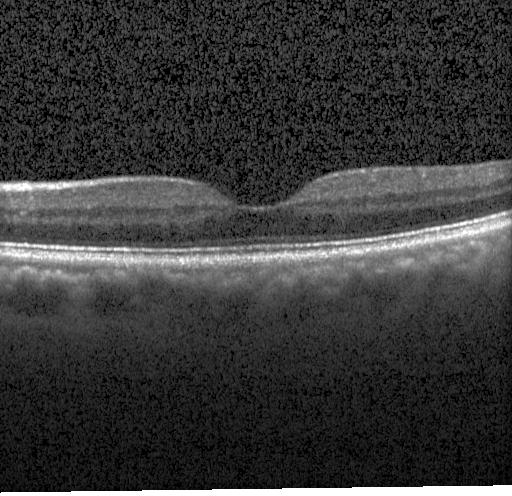

OCT B-scan · fovea-centered · instrument: Heidelberg Spectralis. Impression: no choroidal neovascularization, diabetic macular edema, or drusen.